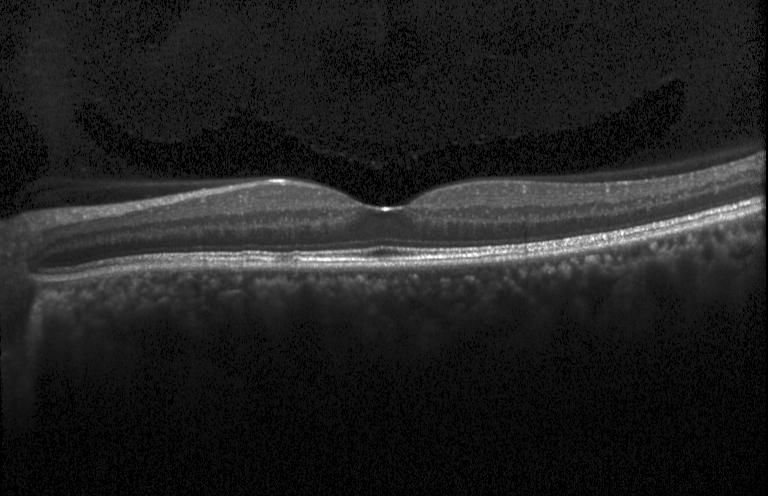 Acquired on a Heidelberg Spectralis, retinal OCT B-scan, SD-OCT, through the macula — This B-scan demonstrates neither CNV, DME, nor drusen.